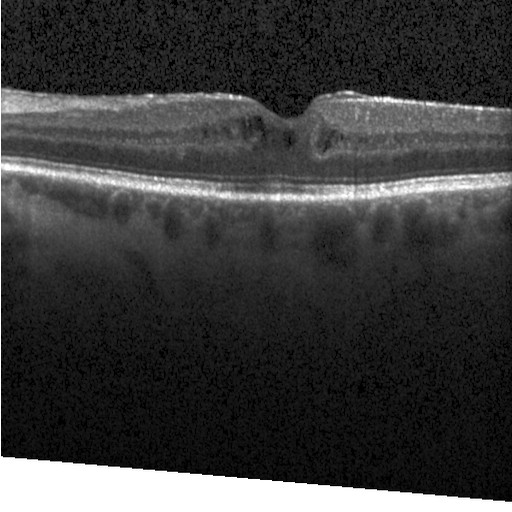

Optical coherence tomography scan. Instrument: Heidelberg Spectralis. Spectral-domain optical coherence tomography — Finding: diabetic macular edema.